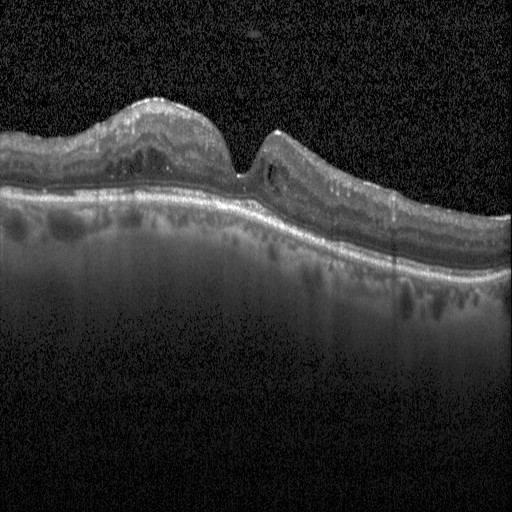 Optical coherence tomography B-scan · spectral-domain optical coherence tomography
Dx: diabetic macular edema (DME).